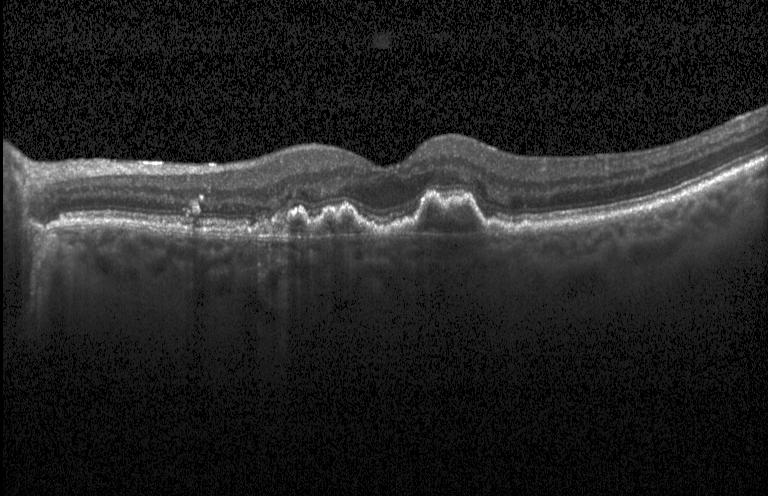 This B-scan demonstrates a choroidal neovascular membrane.